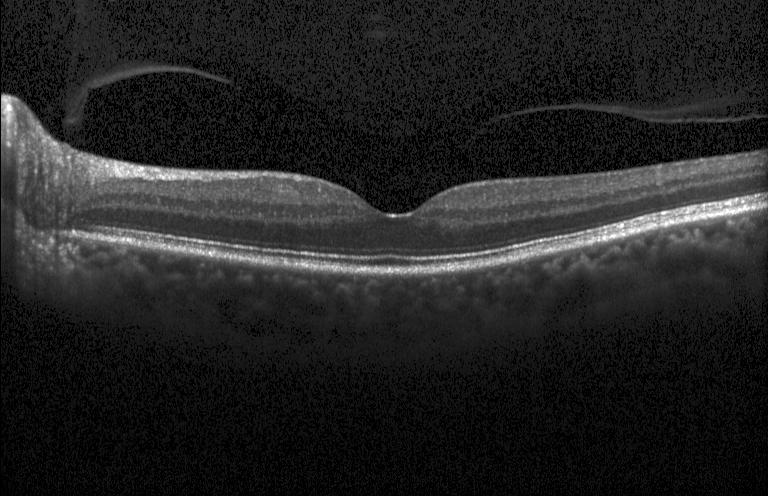 OCT B-scan — Finding: neither choroidal neovascularization, diabetic macular edema, nor drusen.